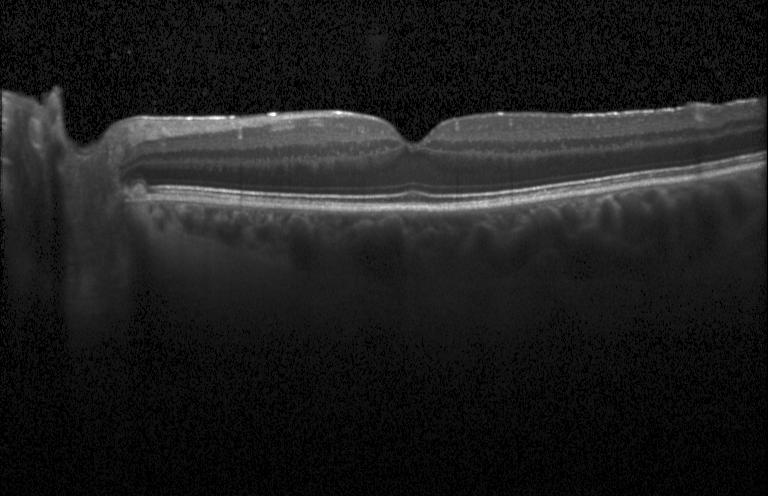 The scan shows no choroidal neovascularization, no diabetic macular edema, and no drusen.